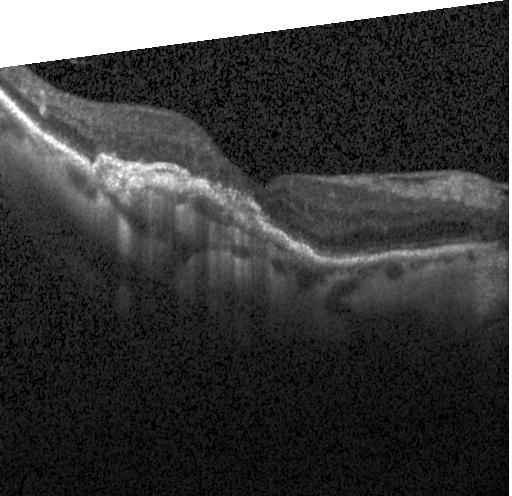

Fovea-centered · spectral-domain optical coherence tomography · instrument: Heidelberg Spectralis · retinal OCT B-scan. Choroidal neovascularization.